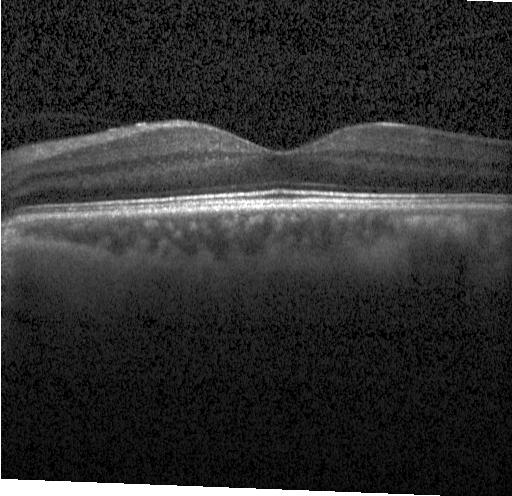 Optical coherence tomography B-scan
Diagnosis: no evidence of choroidal neovascularization, diabetic macular edema, or drusen.